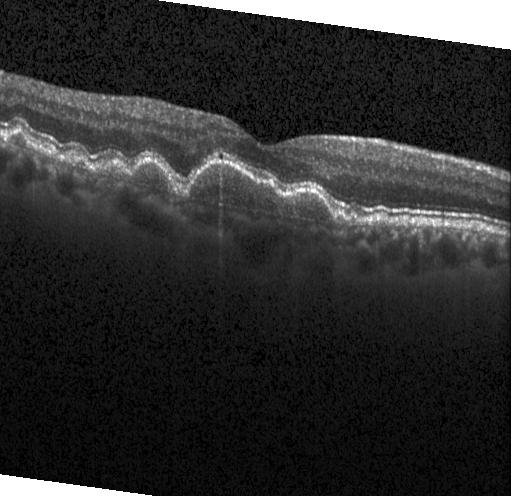
Impression: sub-RPE drusenoid deposits.